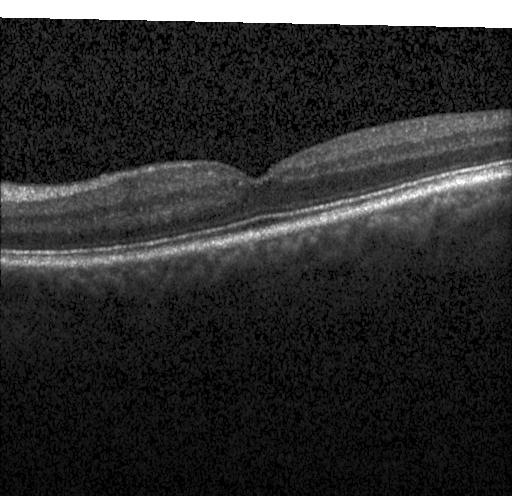 Impression: no evidence of CNV, DME, or drusen.